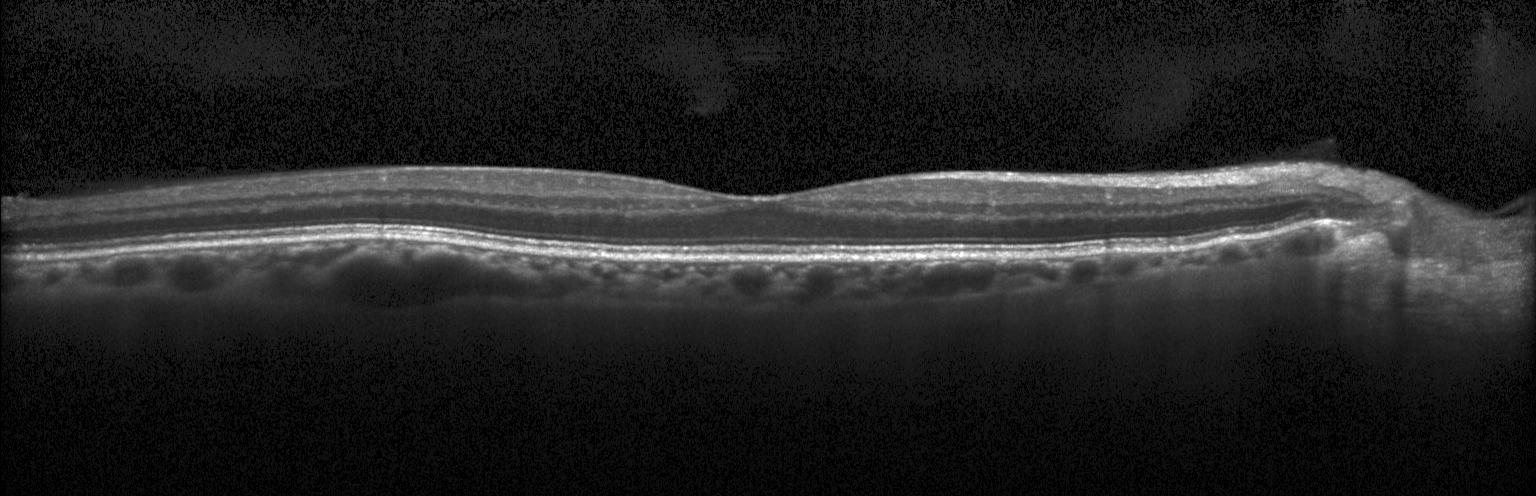
Retinal OCT B-scan, centered on the fovea, instrument: Heidelberg Spectralis. This B-scan demonstrates no choroidal neovascularization, diabetic macular edema, or drusen.